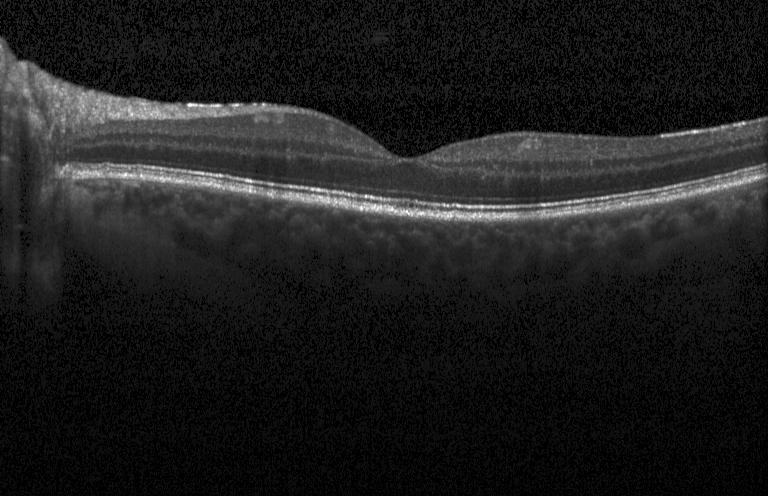

Optical coherence tomography B-scan. Impression: no CNV, DME, or drusen.